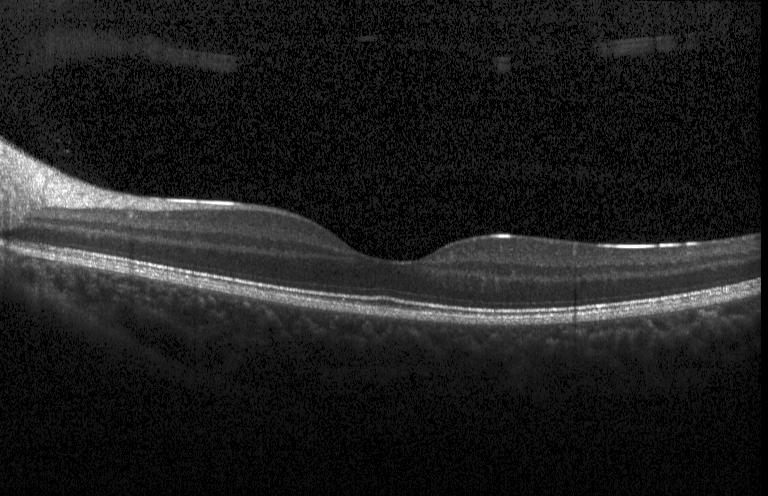

SD-OCT. Optical coherence tomography scan. Instrument: Heidelberg Spectralis. Through the macula
This B-scan demonstrates no choroidal neovascularization, diabetic macular edema, or drusen.